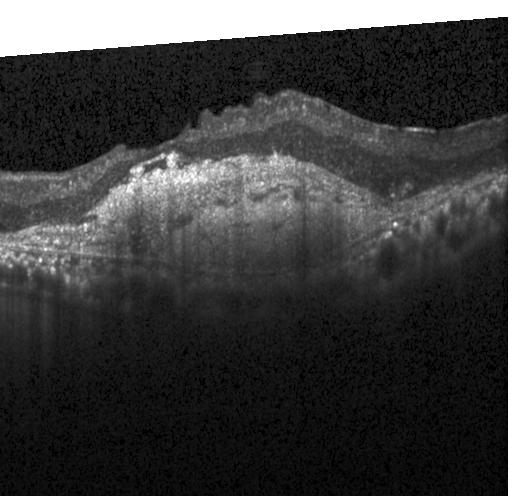 OCT B-scan. Instrument: Heidelberg Spectralis. Horizontal scan through the fovea. Spectral-domain OCT
Diagnosis: CNV.